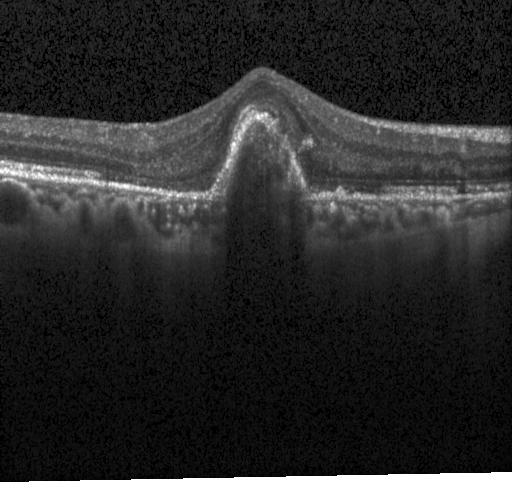 Retinal OCT cross-section · Heidelberg Spectralis OCT system.
Impression: a choroidal neovascular membrane.